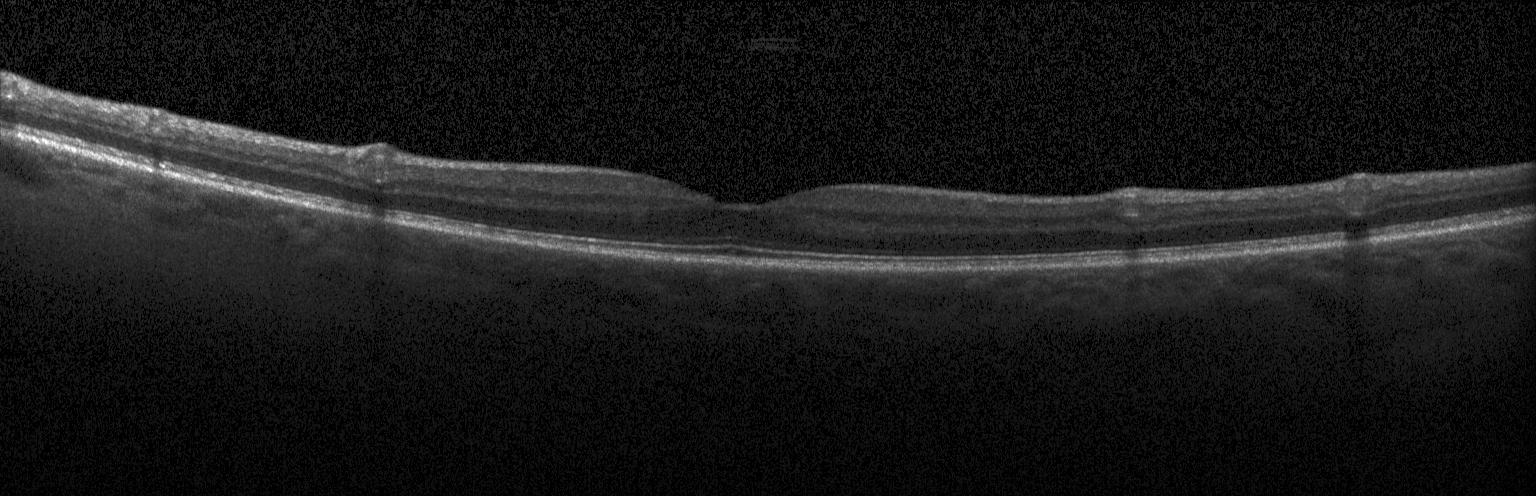

Finding: neither choroidal neovascularization, diabetic macular edema, nor drusen.